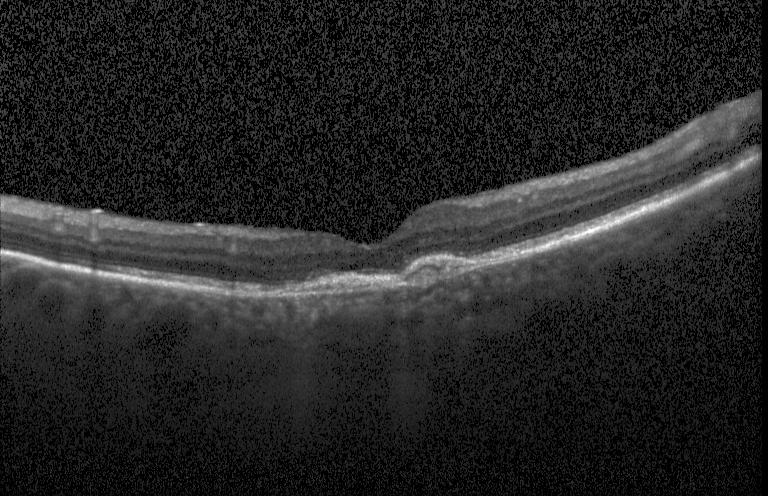
OCT line scan, spectral-domain optical coherence tomography — OCT finding: choroidal neovascularization (CNV).